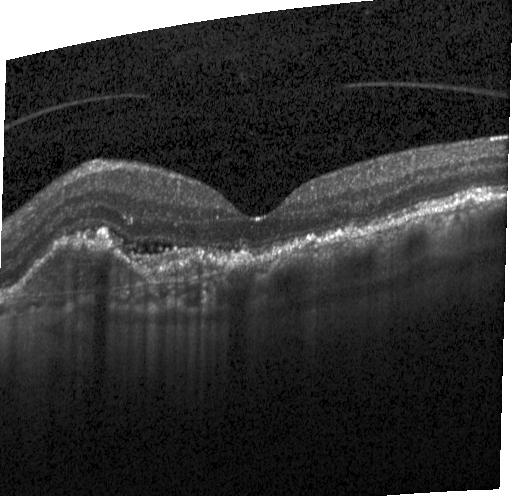

Centered on the fovea, optical coherence tomography scan. This B-scan demonstrates a choroidal neovascular membrane.